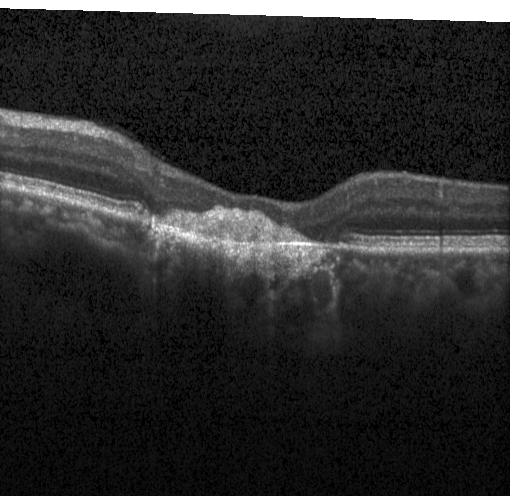 OCT B-scan — Assessment: a choroidal neovascular membrane.